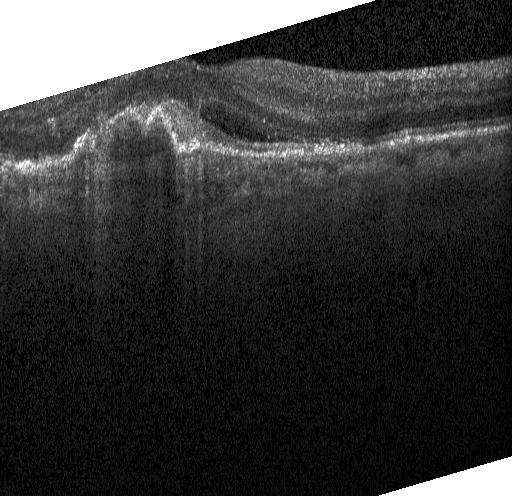 Assessment: a choroidal neovascular membrane.